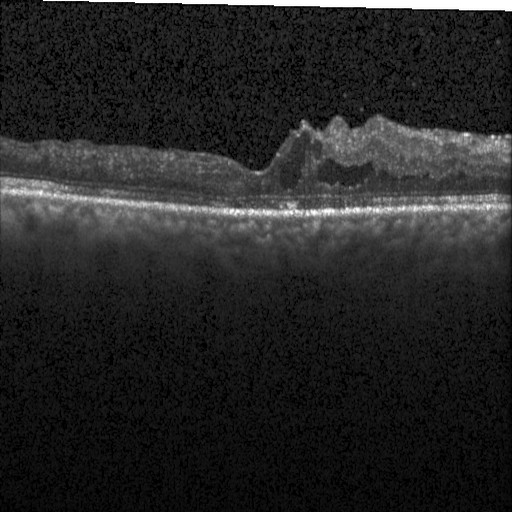

Optical coherence tomography scan
Assessment: diabetic macular edema (DME).